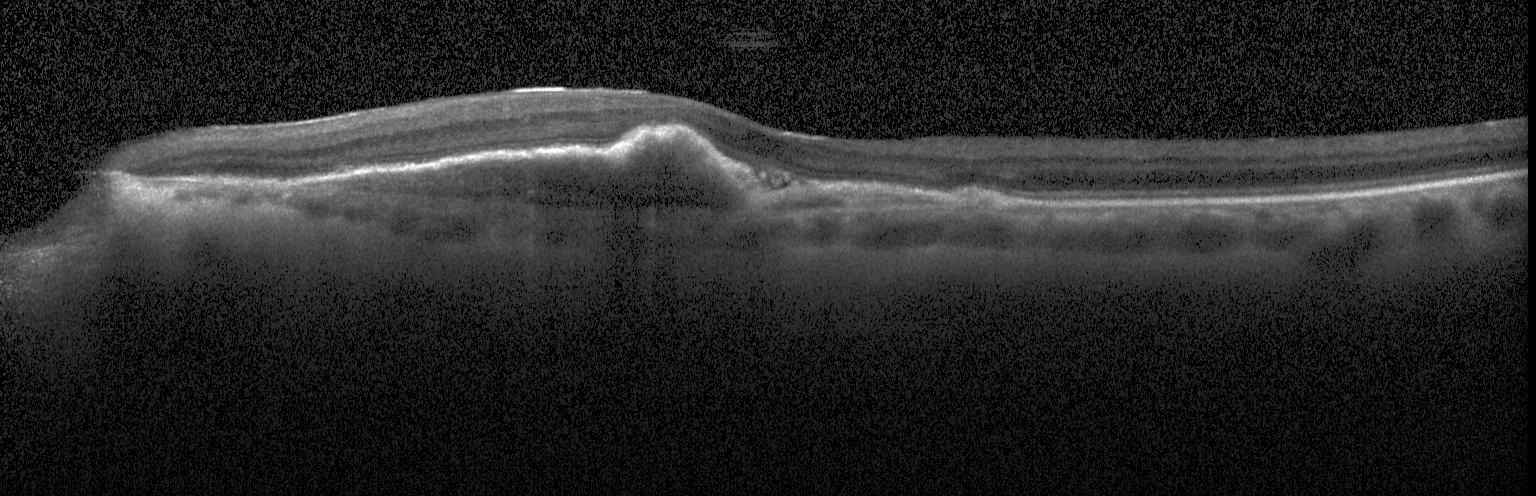

This B-scan demonstrates a choroidal neovascular membrane.